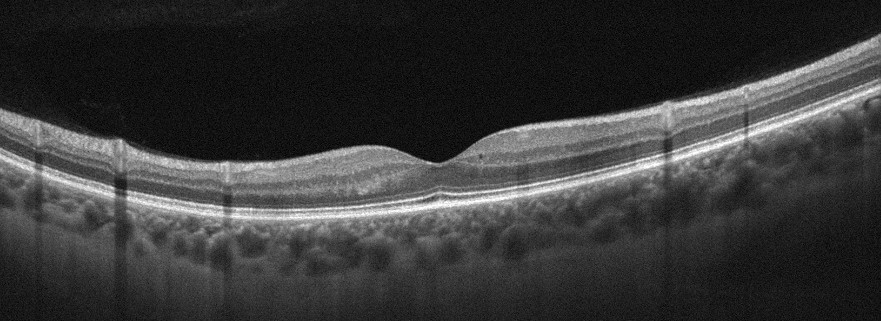 Macular OCT: absence of AMD, DME, ERM, RAO, RVO, and vitreomacular interface disease.